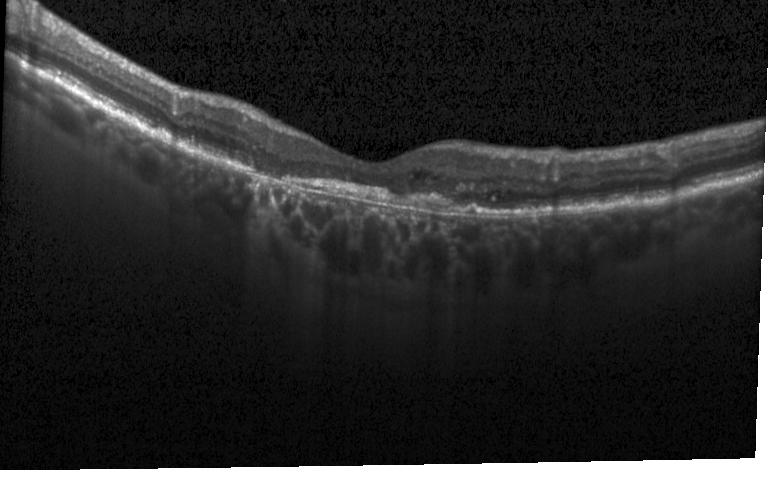 Retinal OCT B-scan · spectral-domain OCT · acquired on a Heidelberg Spectralis. Diagnosis: CNV.